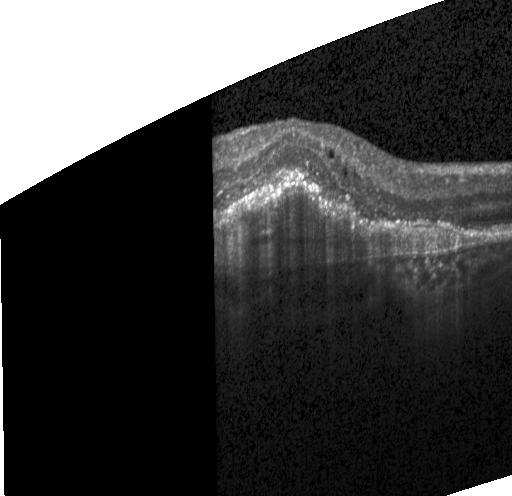 Impression: a choroidal neovascular membrane.